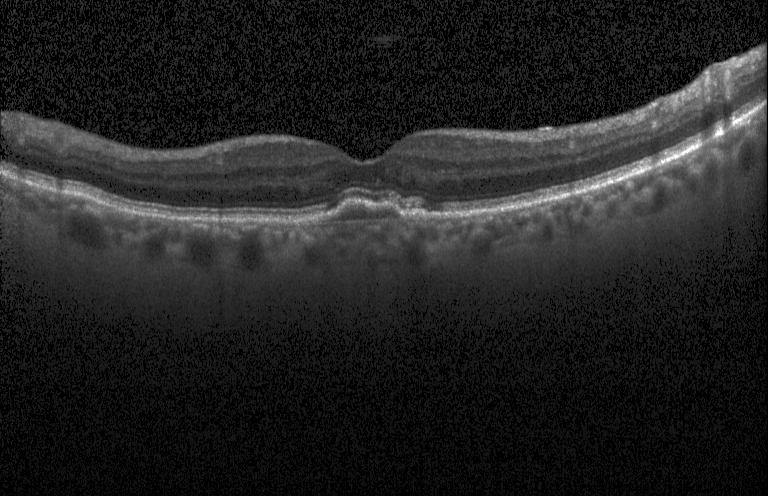

Heidelberg Spectralis · spectral-domain OCT · through the macula · optical coherence tomography B-scan — Finding: choroidal neovascularization (CNV).